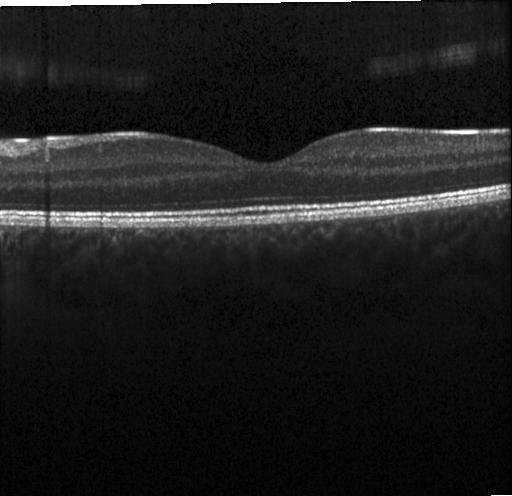

Optical coherence tomography B-scan.
This B-scan demonstrates no CNV, no DME, and no drusen.